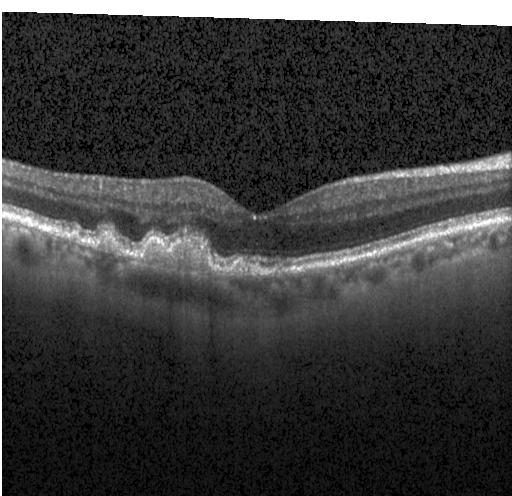
OCT line scan — Dx: sub-RPE drusenoid deposits.